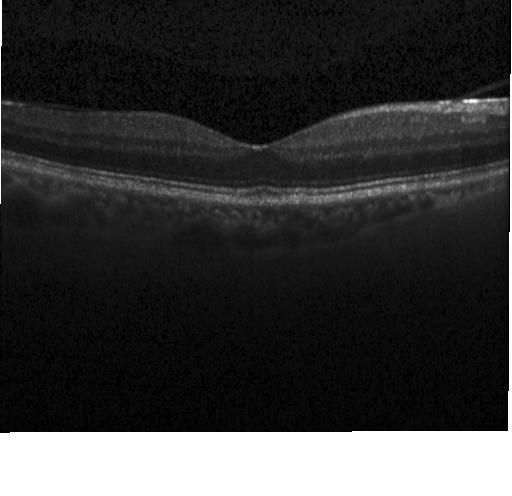
Heidelberg Spectralis · retinal OCT B-scan · SD-OCT · centered on the fovea
Diagnosis: no choroidal neovascularization, no diabetic macular edema, and no drusen.